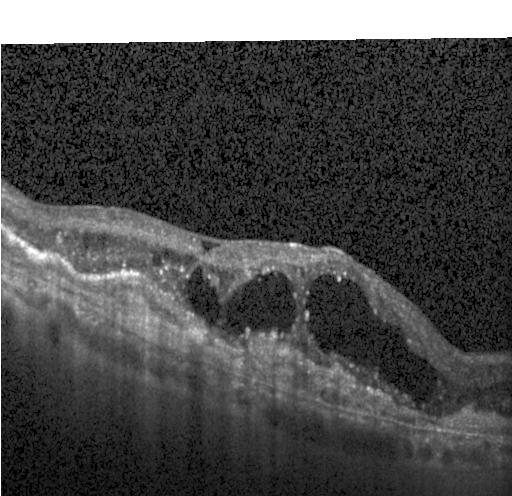

Finding: a choroidal neovascular membrane.